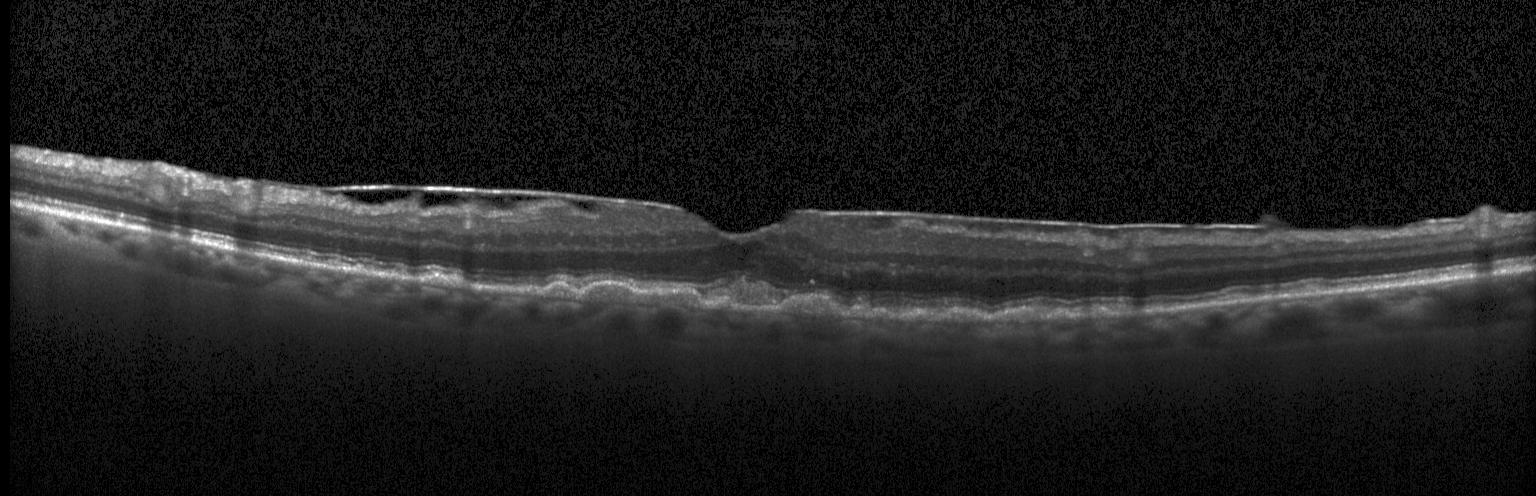
OCT finding: drusen.